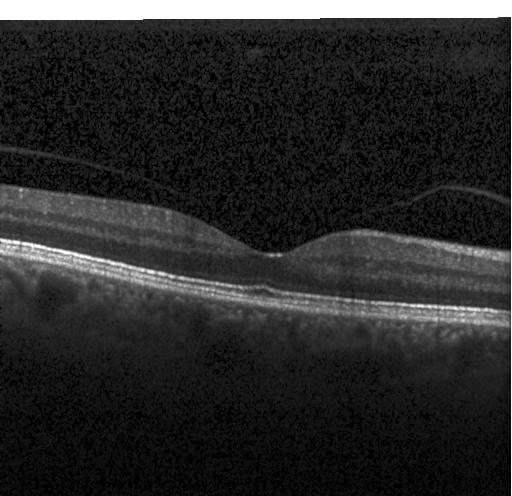

OCT line scan · spectral-domain OCT. Macular OCT: no choroidal neovascularization, no diabetic macular edema, and no drusen.